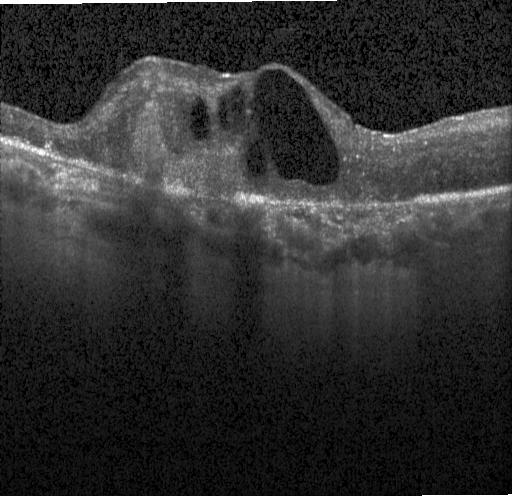

Spectral-domain OCT B-scan: a choroidal neovascular membrane.